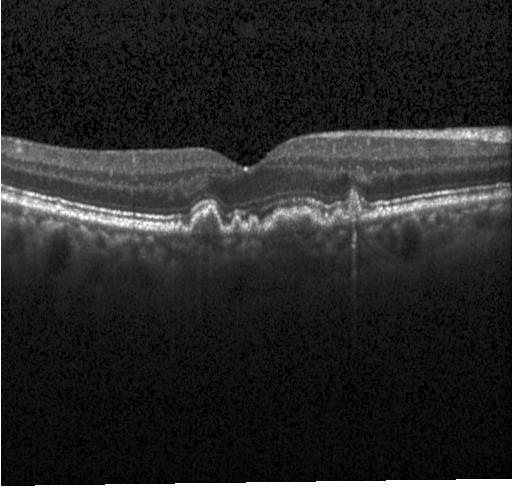 Diagnosis: sub-RPE drusenoid deposits.